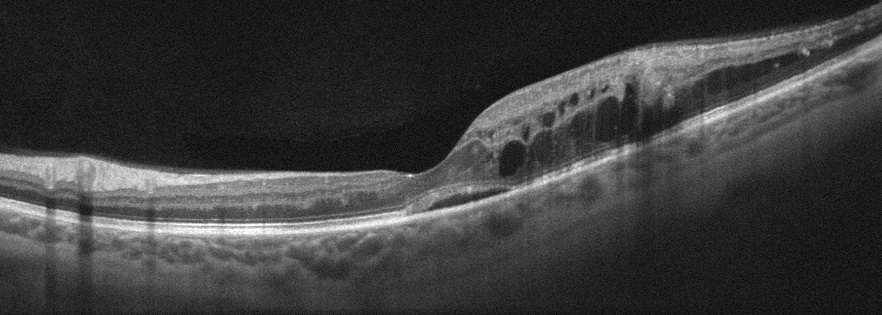
Fovea-centered, Optovue Avanti RTVue XR, OCT line scan. This B-scan demonstrates retinal vein occlusion (RVO).